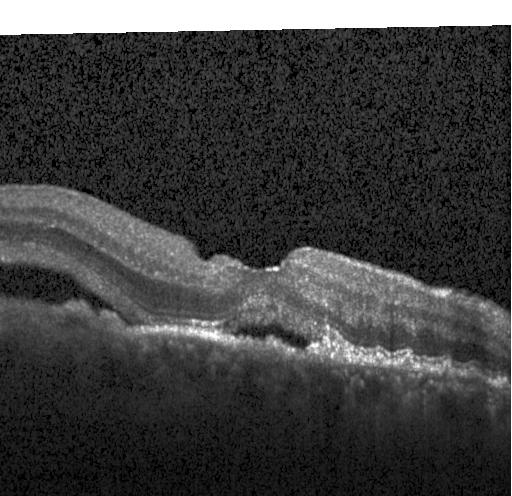
Through the macula · spectral-domain OCT · optical coherence tomography B-scan · Heidelberg Spectralis OCT system
Impression: choroidal neovascularization (CNV).